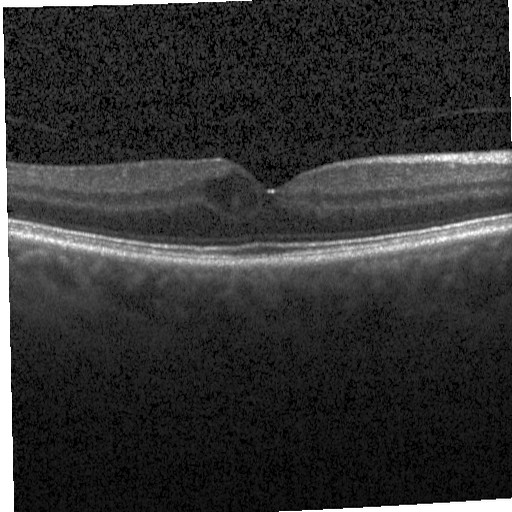
Retinal OCT B-scan · horizontal scan through the fovea.
Dx: DME.